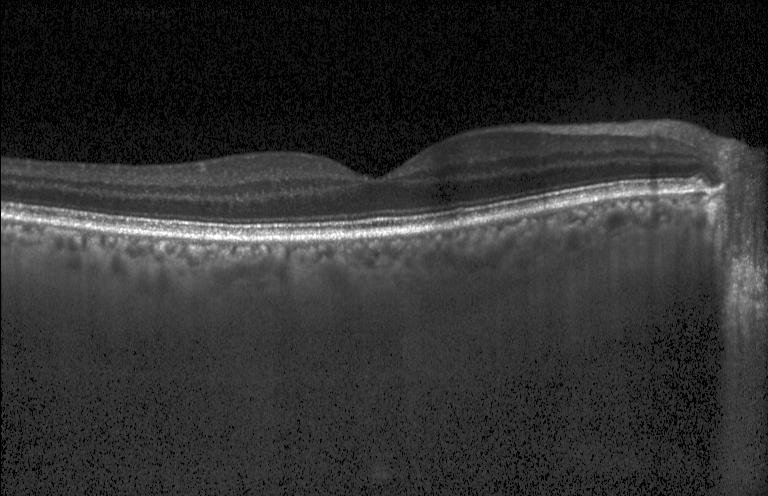

Assessment: no choroidal neovascularization, diabetic macular edema, or drusen.